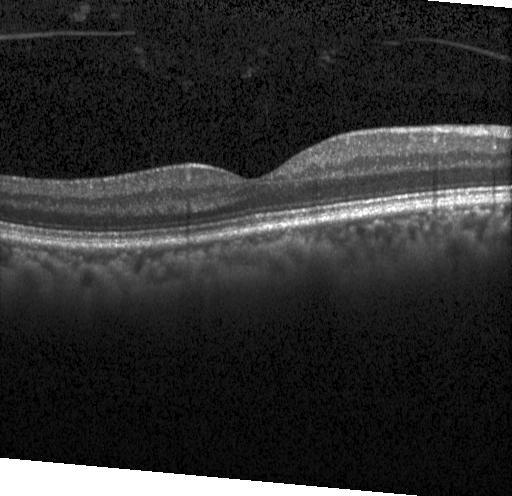

Spectral-domain OCT, retinal OCT B-scan, macular scan, instrument: Heidelberg Spectralis — OCT finding: neither choroidal neovascularization, diabetic macular edema, nor drusen.